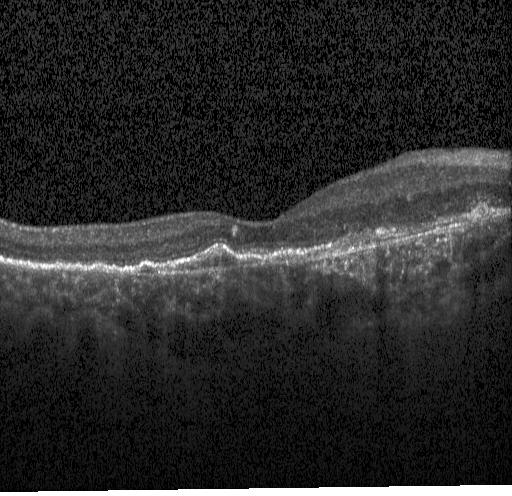

OCT line scan. Fovea-centered
Impression: a choroidal neovascular membrane.